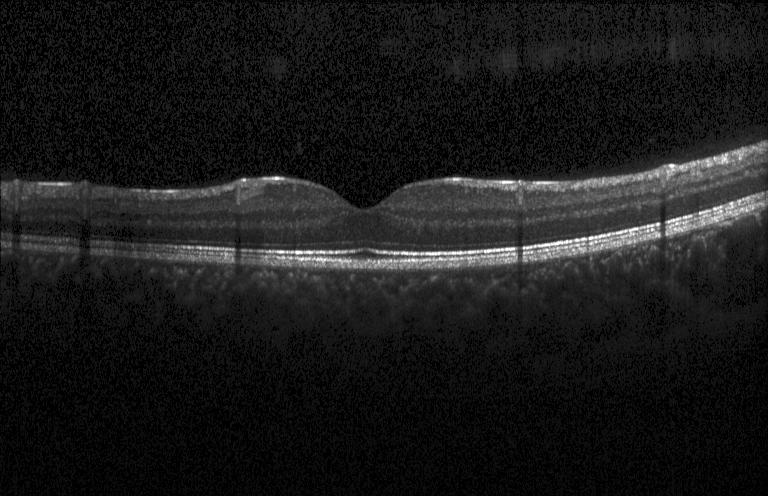 Retinal OCT cross-section — Diagnosis: neither CNV, DME, nor drusen.